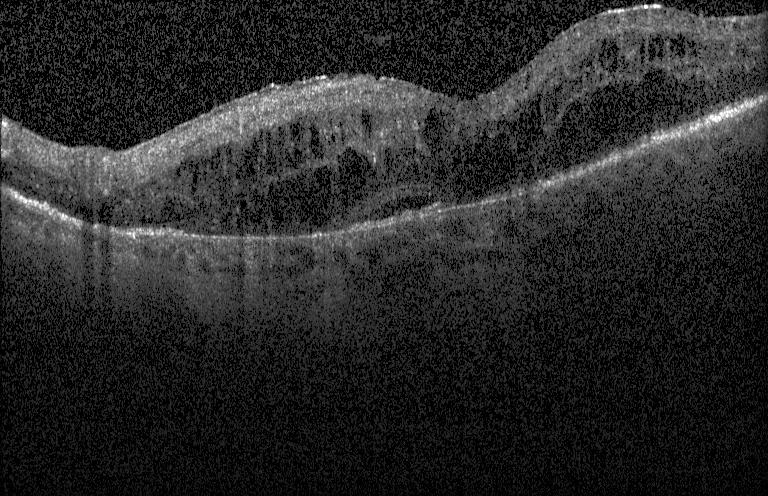 Acquired on a Heidelberg Spectralis; retinal OCT cross-section; through the macula; spectral-domain optical coherence tomography — Diagnosis: CNV.